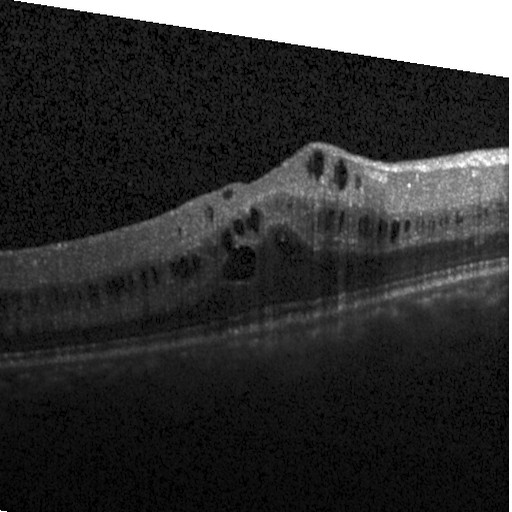
Impression: diabetic macular edema (DME).